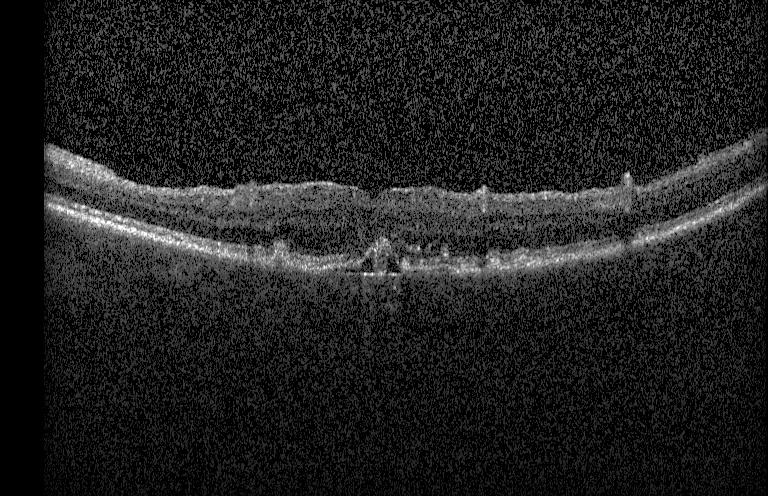

Macular scan, spectral-domain optical coherence tomography, OCT line scan. Macular OCT: a choroidal neovascular membrane.